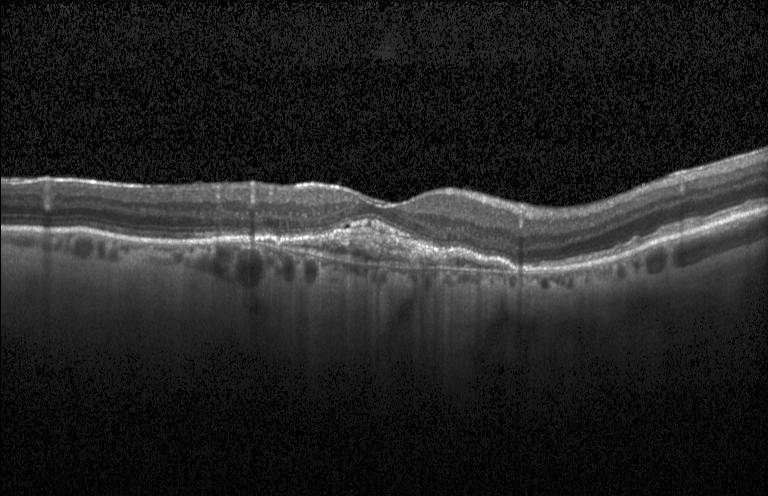

Retinal OCT cross-section showing CNV.